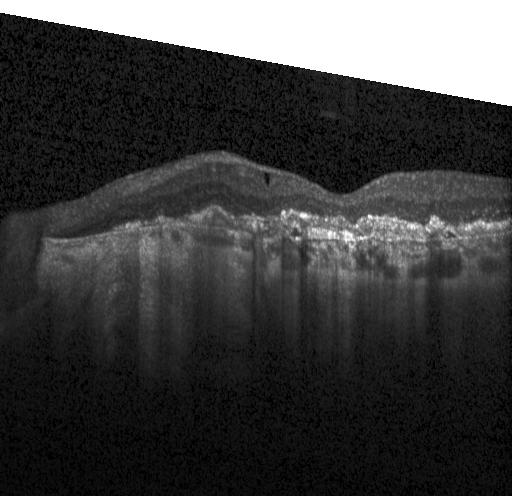
Retinal OCT B-scan. Heidelberg Spectralis OCT system — Diagnosis: choroidal neovascularization (CNV).